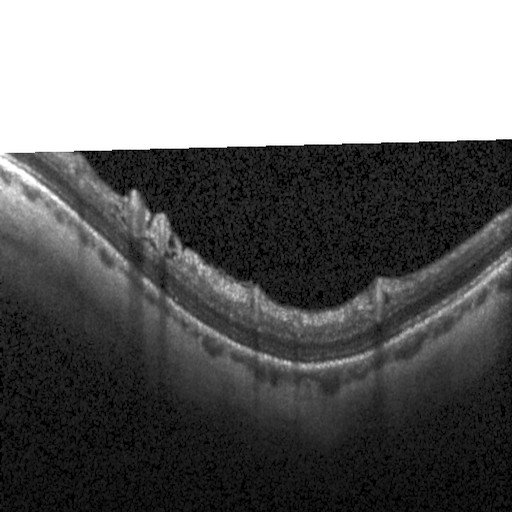 Assessment: diabetic macular edema.